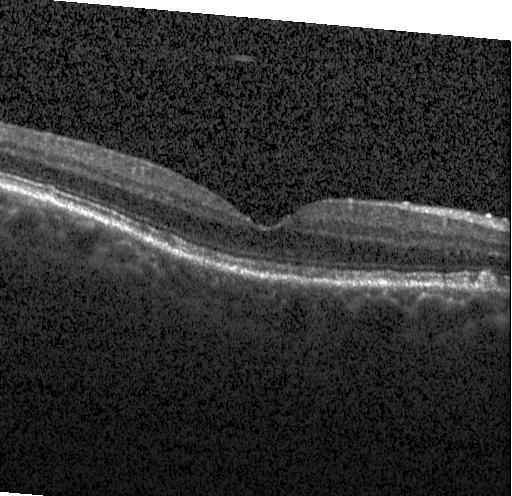
Impression: drusen.